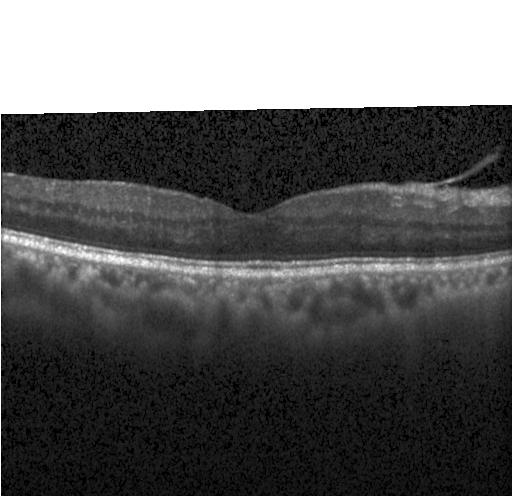

Retinal OCT cross-section showing neither choroidal neovascularization, diabetic macular edema, nor drusen.